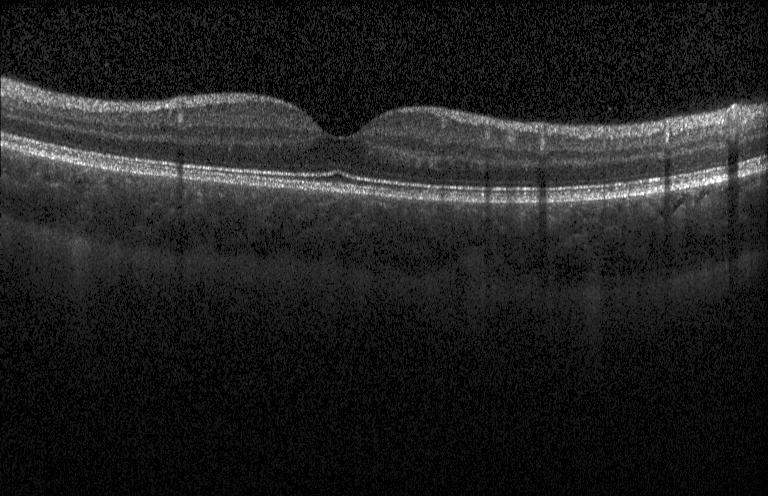 OCT finding: no choroidal neovascularization, diabetic macular edema, or drusen.